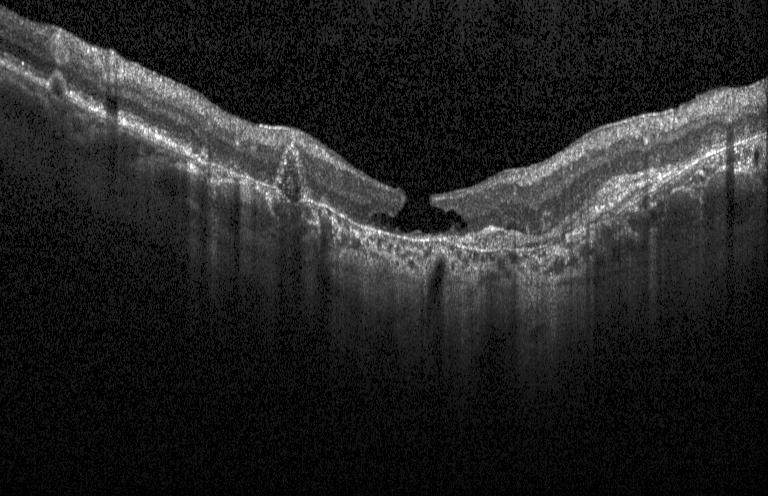

Through the macula; SD-OCT; acquired on a Heidelberg Spectralis; retinal OCT B-scan. Finding: a choroidal neovascular membrane.